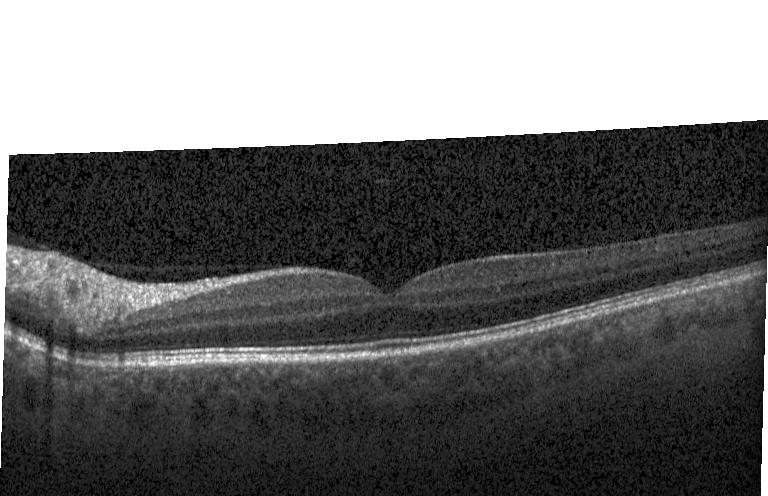
OCT B-scan — Macular OCT: no CNV, DME, or drusen.